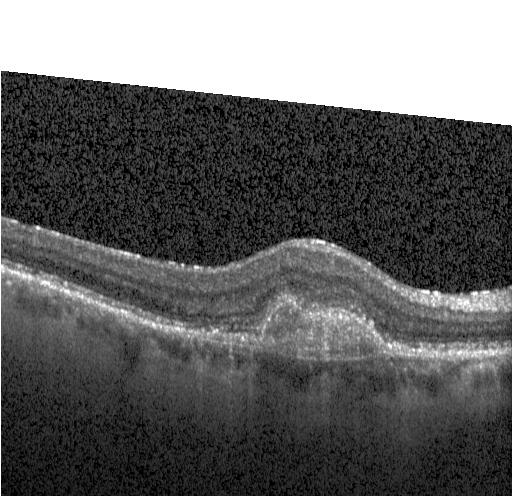

Centered on the fovea; retinal OCT cross-section.
This B-scan demonstrates CNV.